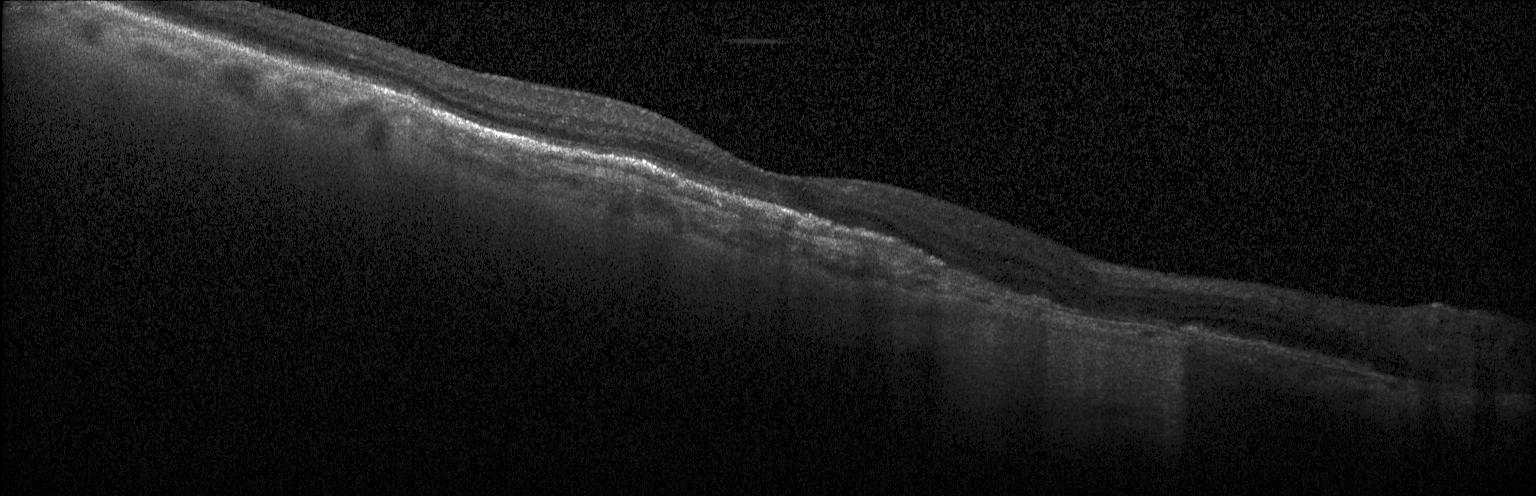
Macular scan. Retinal OCT cross-section. Instrument: Heidelberg Spectralis. Spectral-domain OCT — Finding: a choroidal neovascular membrane.